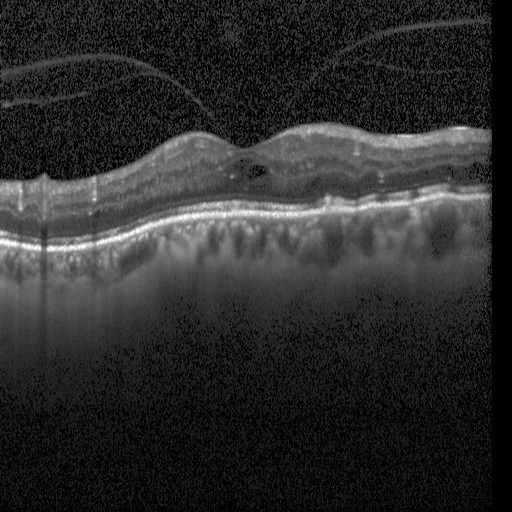

Finding: diabetic macular edema (DME).